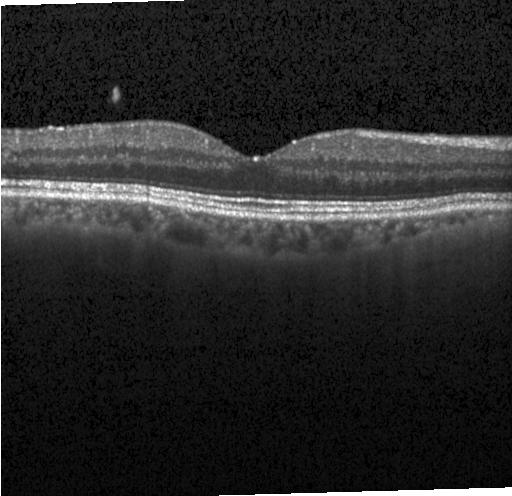 Spectral-domain OCT; optical coherence tomography B-scan; macular scan; instrument: Heidelberg Spectralis
Diagnosis: neither choroidal neovascularization, diabetic macular edema, nor drusen.